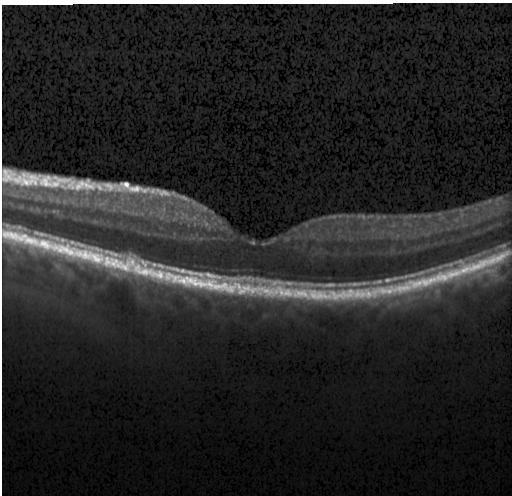 OCT B-scan showing multiple drusen.